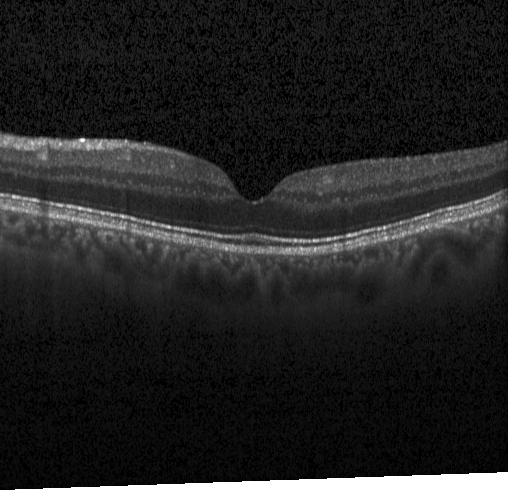

Horizontal scan through the fovea; retinal OCT B-scan; spectral-domain optical coherence tomography; Heidelberg Spectralis OCT system.
Finding: no choroidal neovascularization, diabetic macular edema, or drusen.